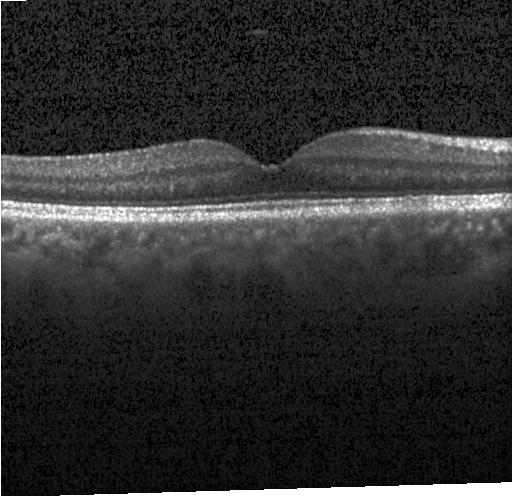 No evidence of choroidal neovascularization, diabetic macular edema, or drusen.